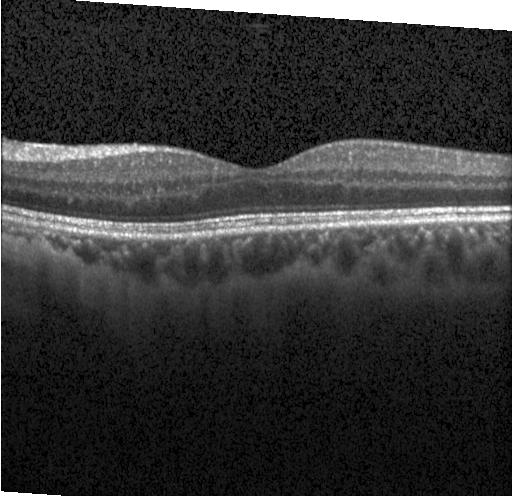
Finding: no choroidal neovascularization, no diabetic macular edema, and no drusen.